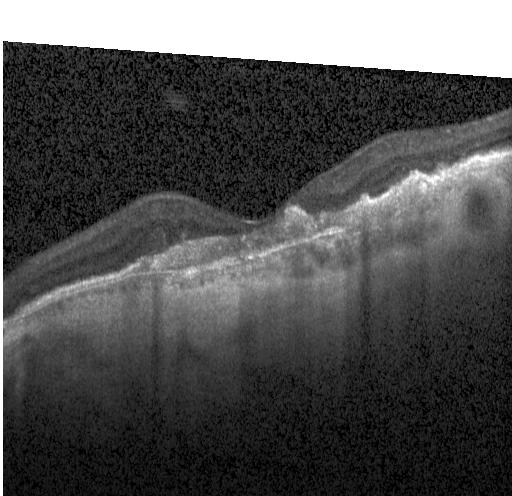
Finding: CNV.